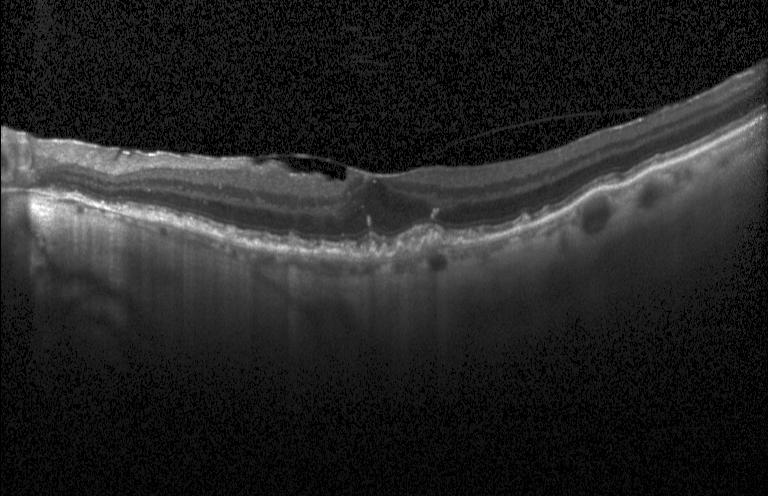

Spectral-domain optical coherence tomography. Optical coherence tomography B-scan. Heidelberg Spectralis OCT system.
Assessment: a choroidal neovascular membrane.